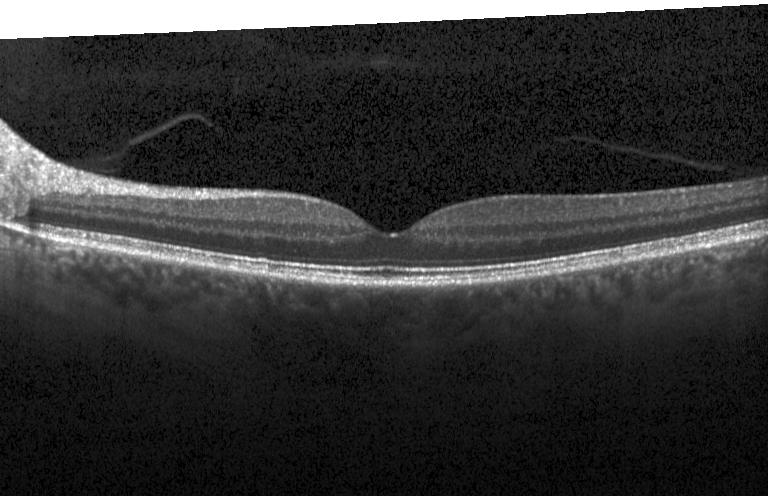 Retinal OCT cross-section.
No choroidal neovascularization, no diabetic macular edema, and no drusen.